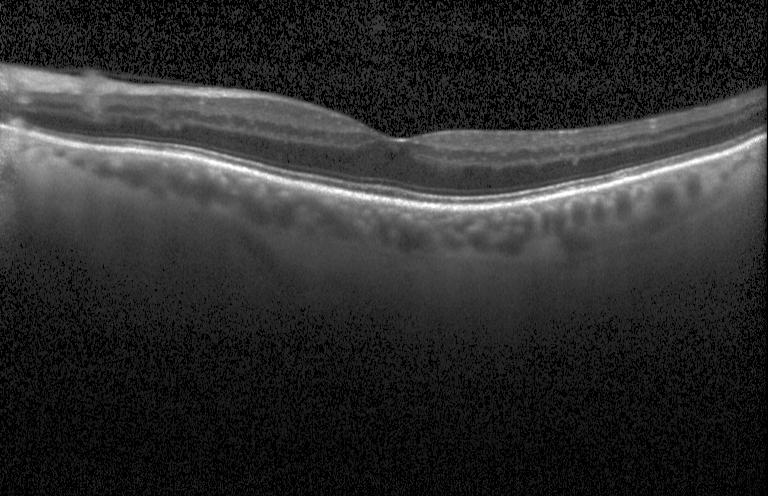

Retinal OCT B-scan. Finding: neither choroidal neovascularization, diabetic macular edema, nor drusen.